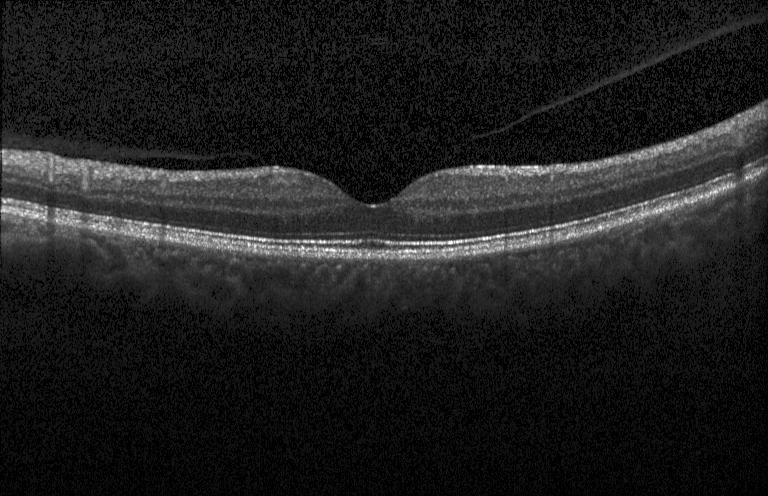

Retinal OCT cross-section · SD-OCT
Dx: no CNV, DME, or drusen.